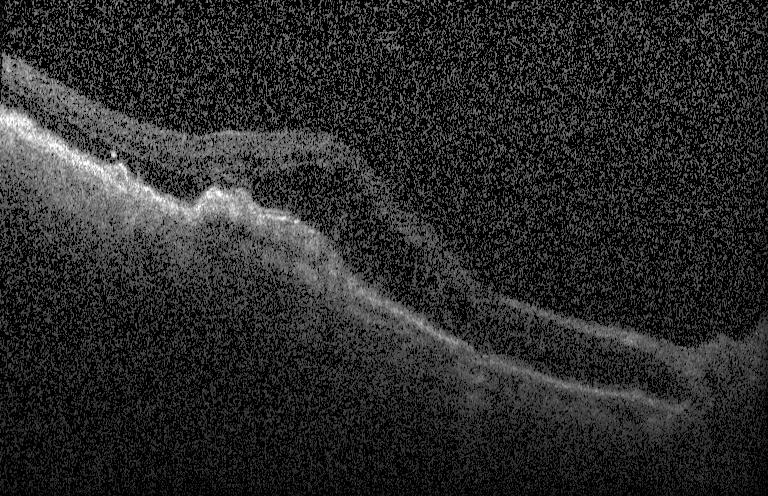 Impression: choroidal neovascularization (CNV).